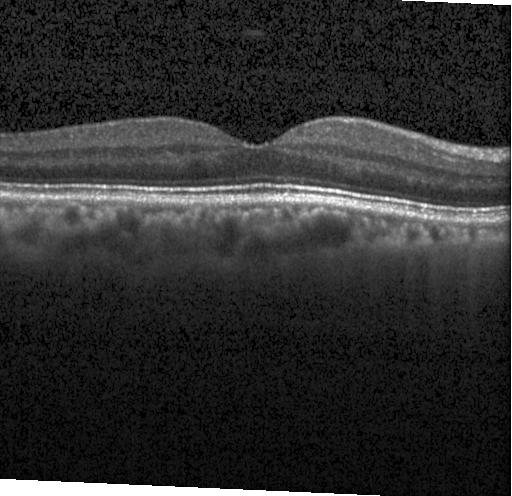
Macular OCT: neither choroidal neovascularization, diabetic macular edema, nor drusen.